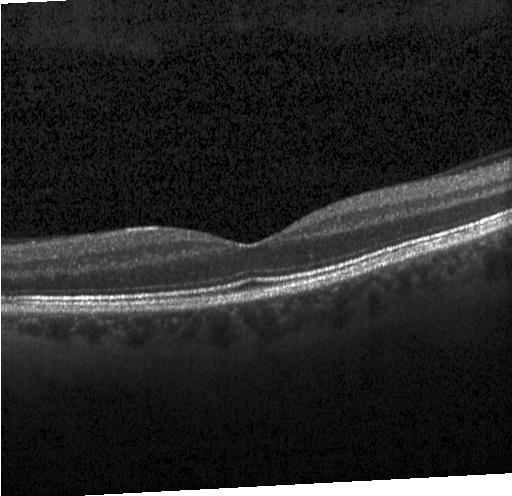
Optical coherence tomography scan. Centered on the fovea. Spectral-domain OCT. Heidelberg Spectralis. Diagnosis: no CNV, DME, or drusen.